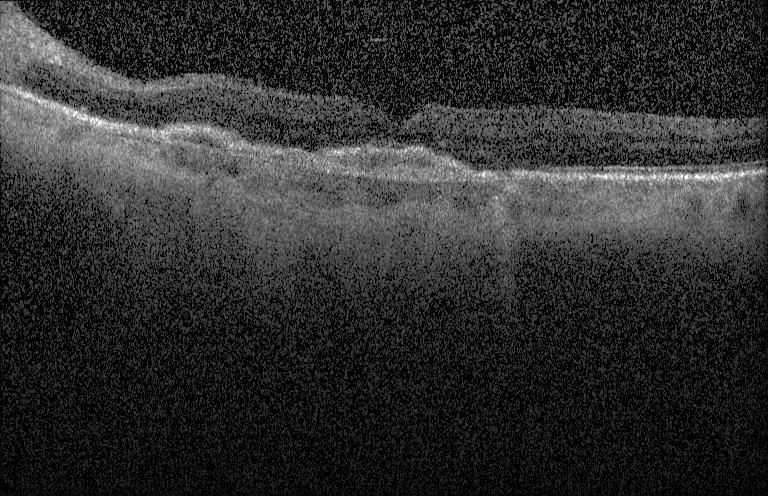

Impression: choroidal neovascularization (CNV).